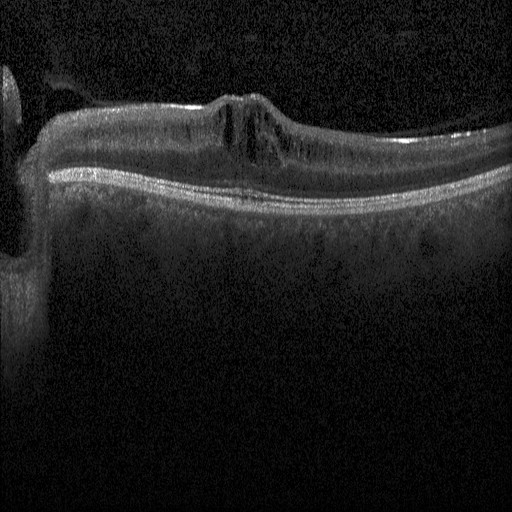 Spectral-domain optical coherence tomography · retinal OCT cross-section. The scan shows DME.